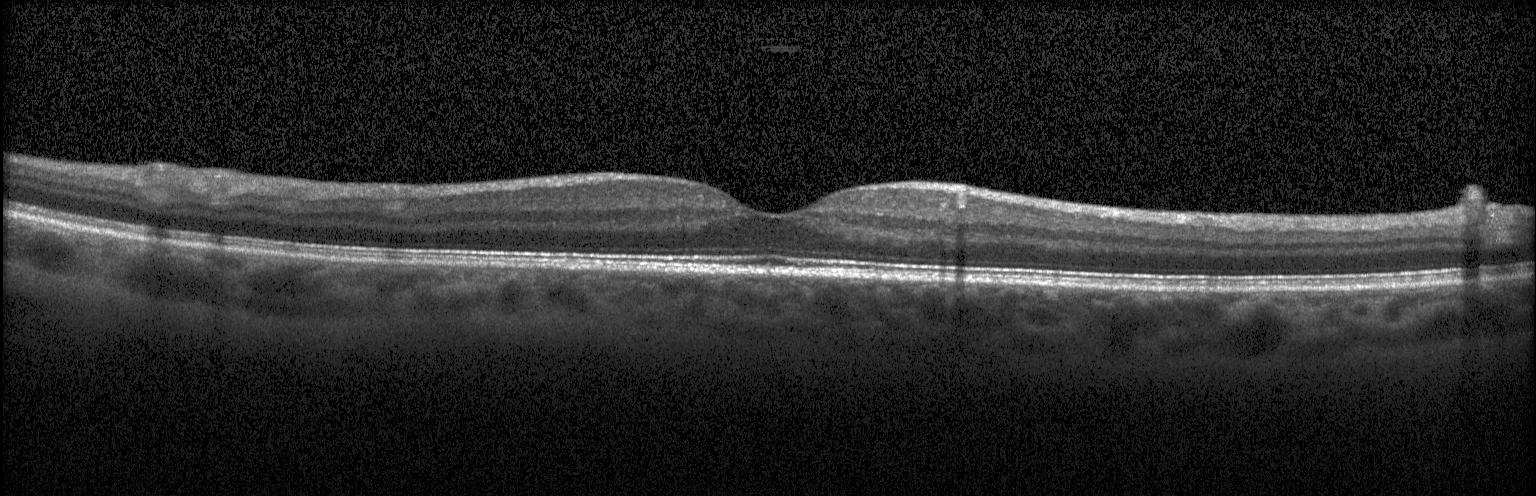
Spectral-domain optical coherence tomography. Retinal OCT cross-section. Centered on the fovea. Instrument: Heidelberg Spectralis. OCT finding: no choroidal neovascularization, no diabetic macular edema, and no drusen.